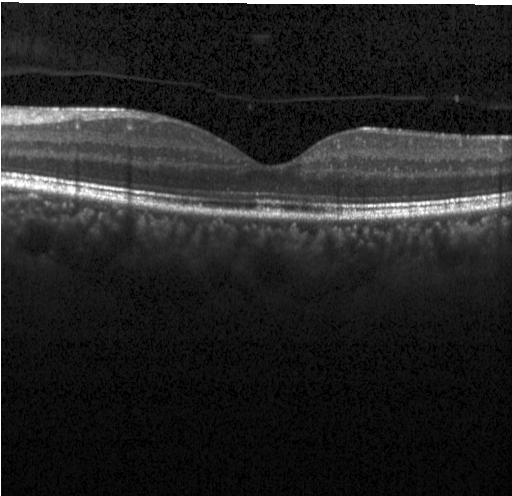

Instrument: Heidelberg Spectralis · SD-OCT · OCT line scan · centered on the fovea
This B-scan demonstrates neither choroidal neovascularization, diabetic macular edema, nor drusen.